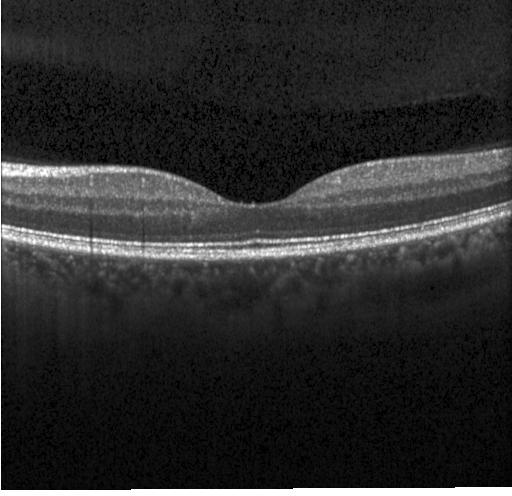
Macular scan. OCT line scan. Heidelberg Spectralis
Assessment: no evidence of choroidal neovascularization, diabetic macular edema, or drusen.